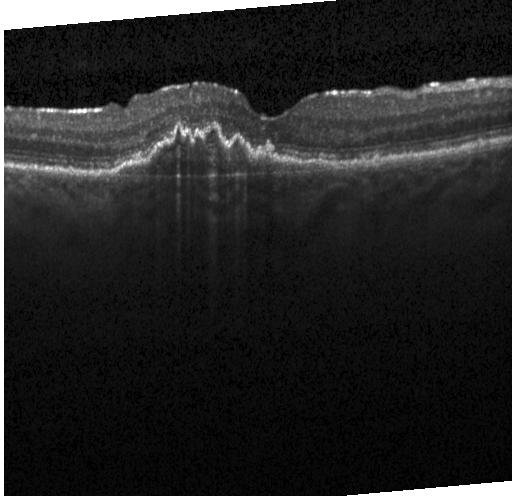
Spectral-domain OCT, fovea-centered, retinal OCT B-scan, Heidelberg Spectralis. Finding: CNV.